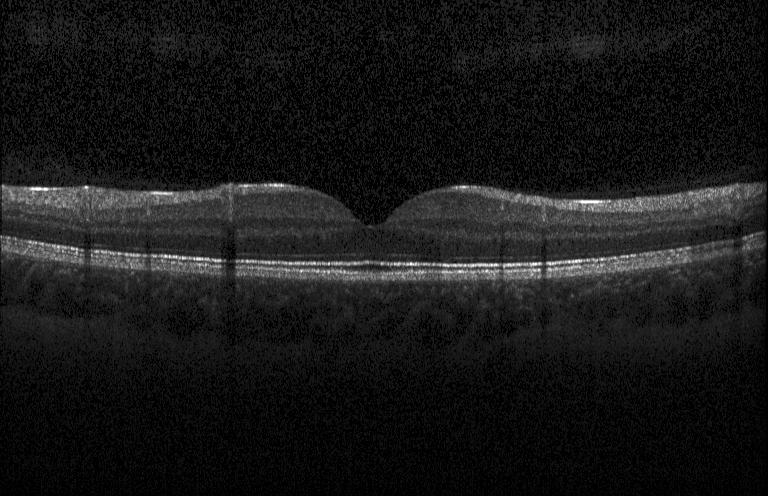
Retinal OCT cross-section. Finding: neither choroidal neovascularization, diabetic macular edema, nor drusen.